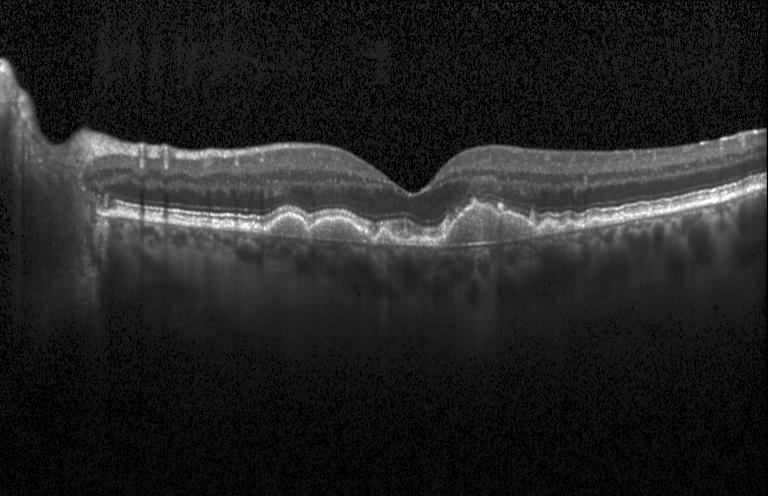 Retinal OCT cross-section
Multiple drusen.